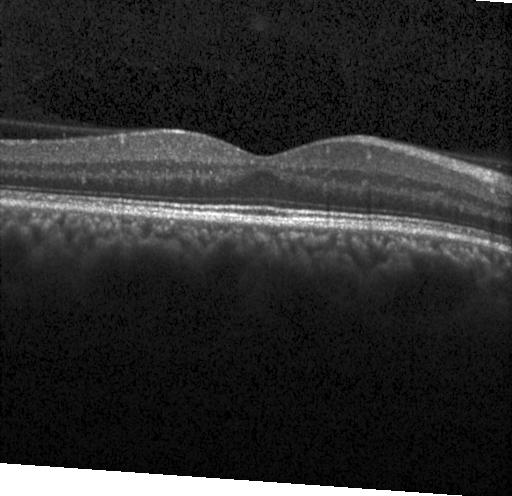

SD-OCT, horizontal scan through the fovea, optical coherence tomography B-scan.
Finding: neither choroidal neovascularization, diabetic macular edema, nor drusen.